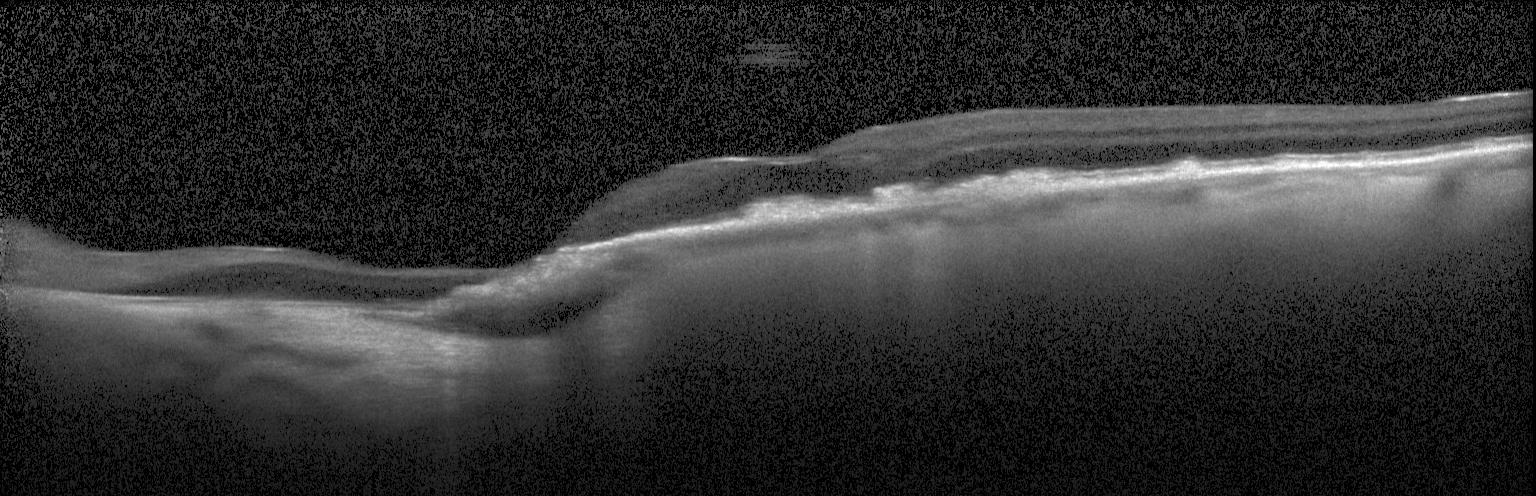

A choroidal neovascular membrane.